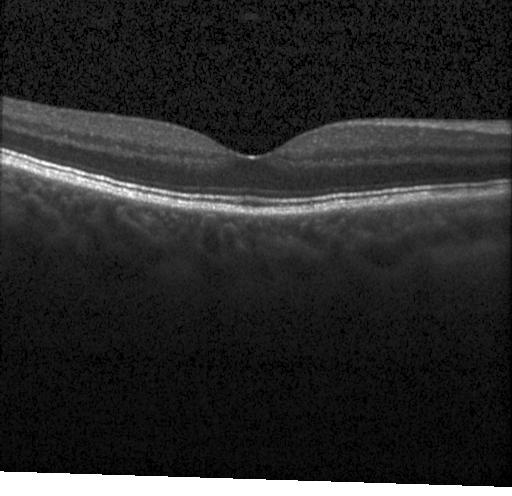 Retinal OCT B-scan
This B-scan demonstrates no choroidal neovascularization, no diabetic macular edema, and no drusen.